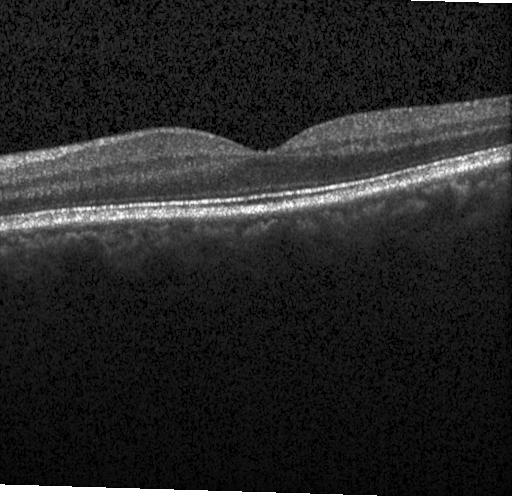
The scan shows no CNV, DME, or drusen.